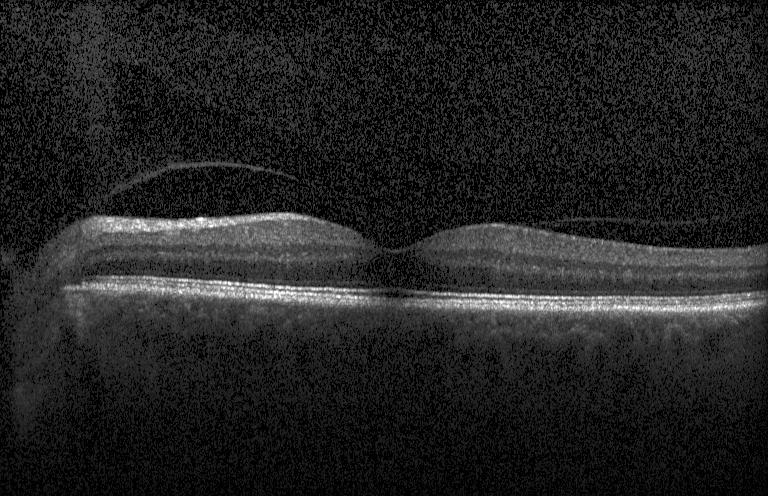
Through the macula. Retinal OCT B-scan
Finding: no evidence of CNV, DME, or drusen.